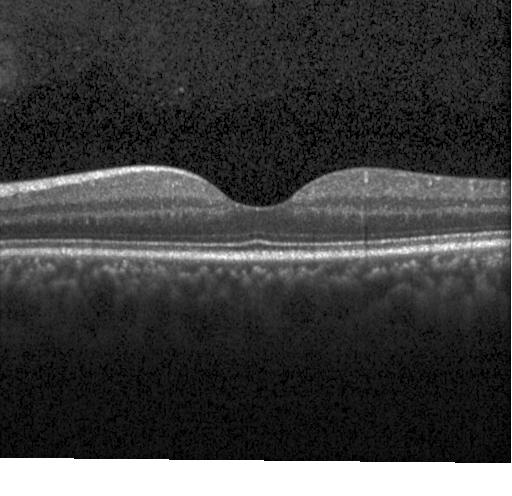
Acquired on a Heidelberg Spectralis; OCT line scan. Assessment: no evidence of CNV, DME, or drusen.